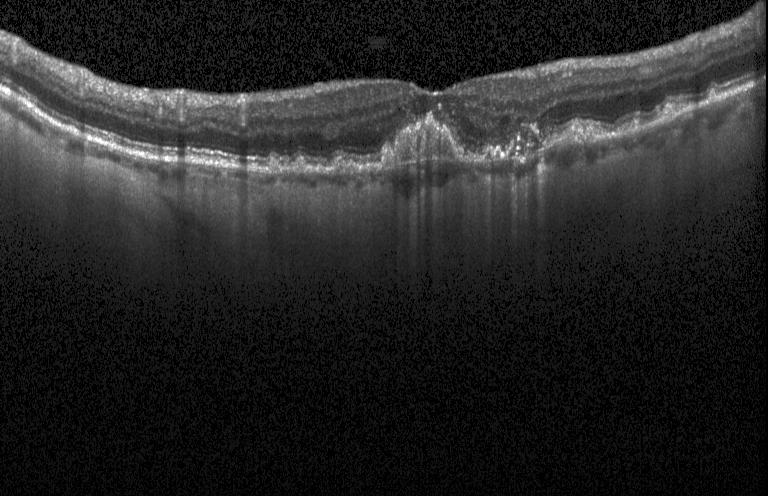

OCT B-scan, spectral-domain optical coherence tomography, acquired on a Heidelberg Spectralis
Dx: choroidal neovascularization.